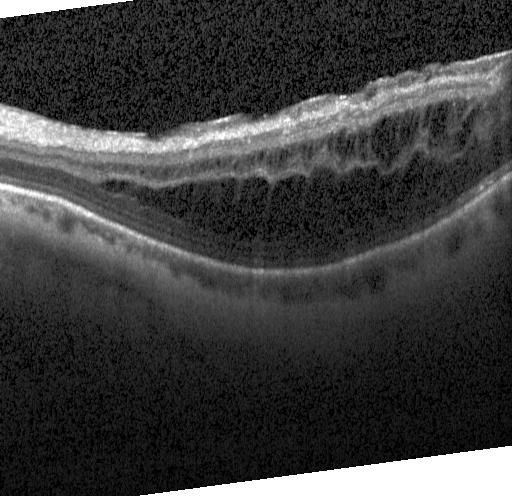 Finding: diabetic macular edema.